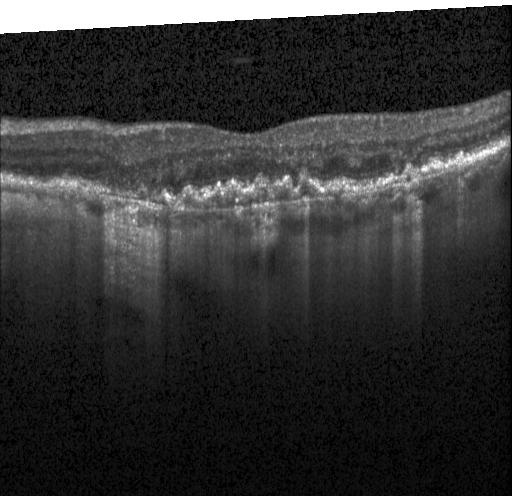
Macular OCT demonstrating CNV.